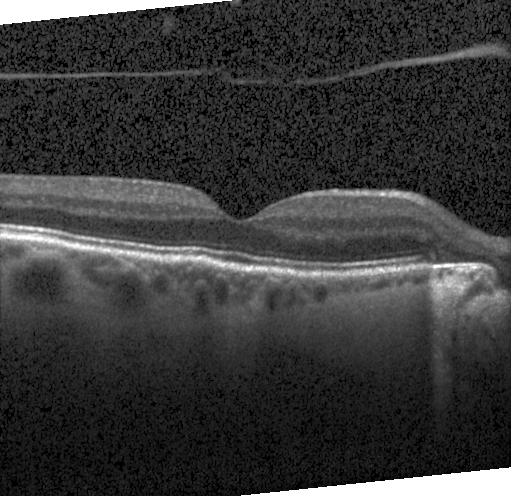 Retinal OCT cross-section.
Assessment: no CNV, DME, or drusen.